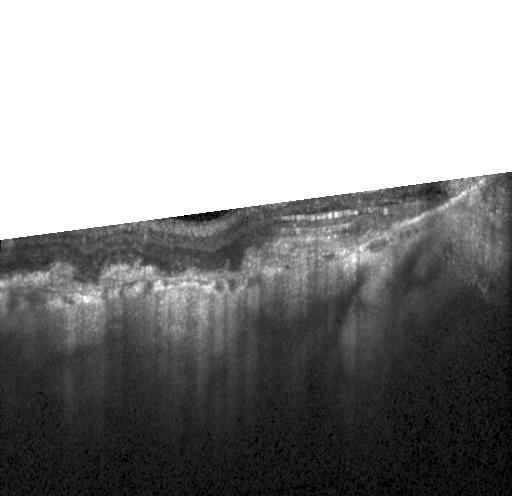 OCT finding: choroidal neovascularization (CNV).